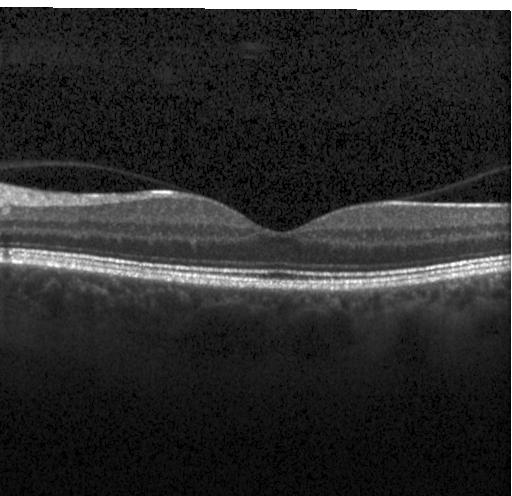
Heidelberg Spectralis; retinal OCT B-scan — Impression: no evidence of choroidal neovascularization, diabetic macular edema, or drusen.